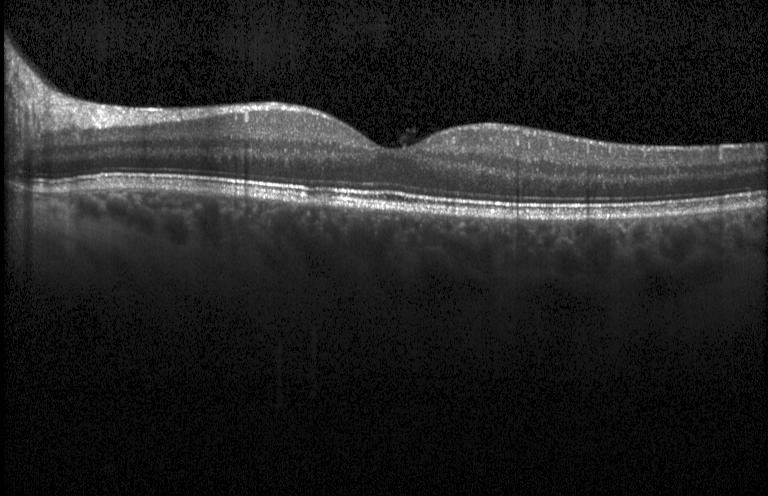 Instrument: Heidelberg Spectralis · retinal OCT B-scan — Impression: neither CNV, DME, nor drusen.